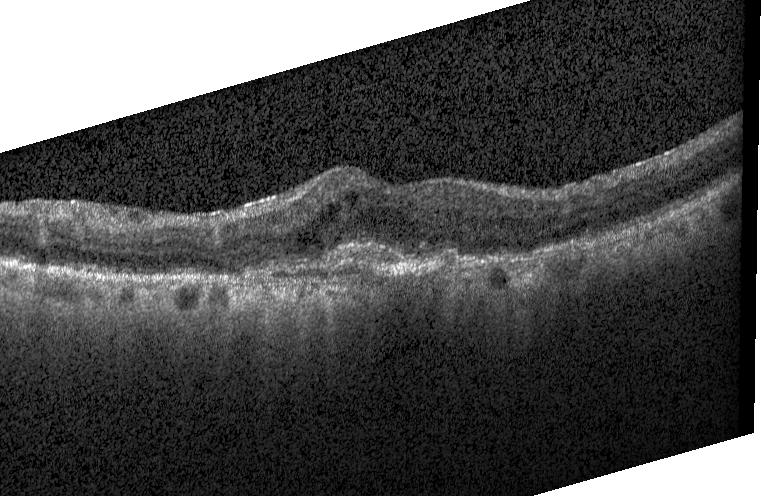 Optical coherence tomography B-scan. Assessment: choroidal neovascularization.